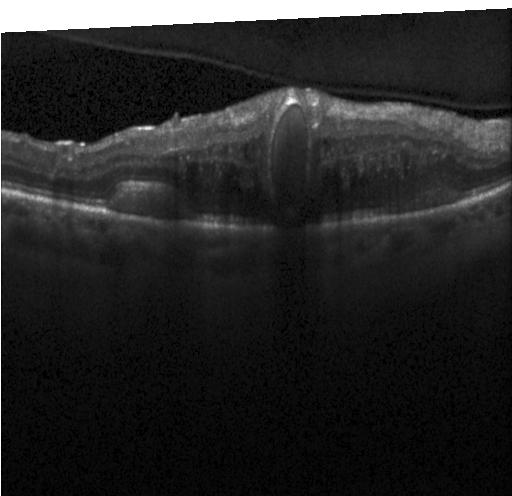
Spectral-domain OCT B-scan: CNV.